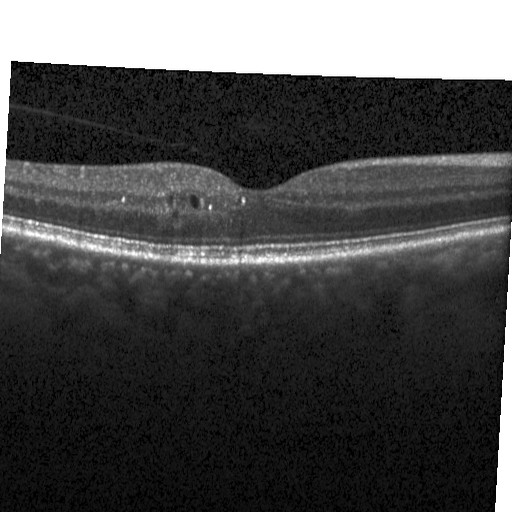 Diagnosis: DME.